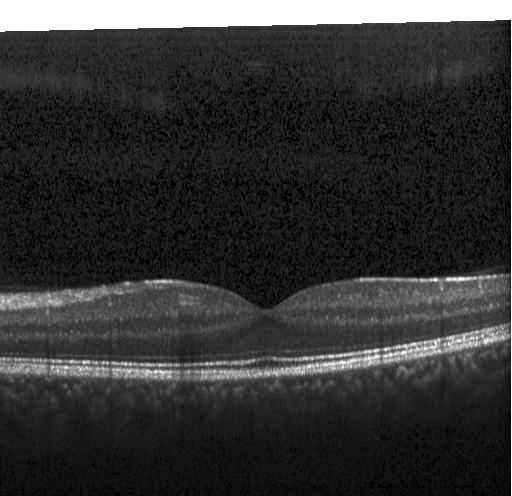 OCT scan showing no evidence of choroidal neovascularization, diabetic macular edema, or drusen.